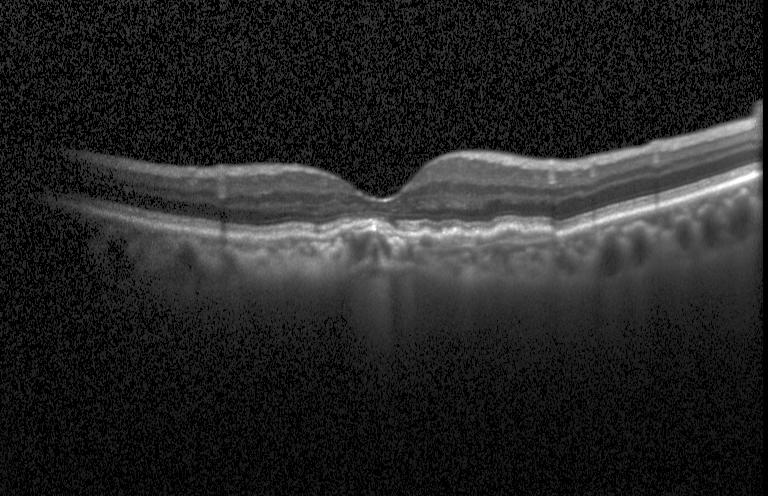 Optical coherence tomography scan
Macular OCT: a choroidal neovascular membrane.